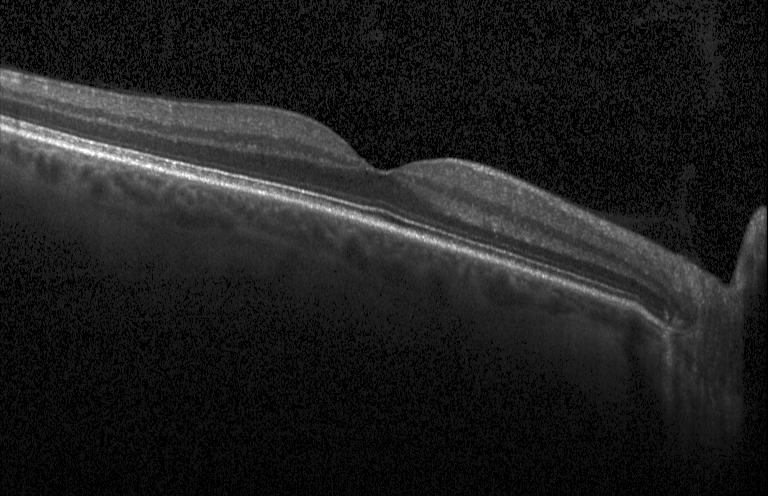
OCT line scan. Finding: no evidence of choroidal neovascularization, diabetic macular edema, or drusen.